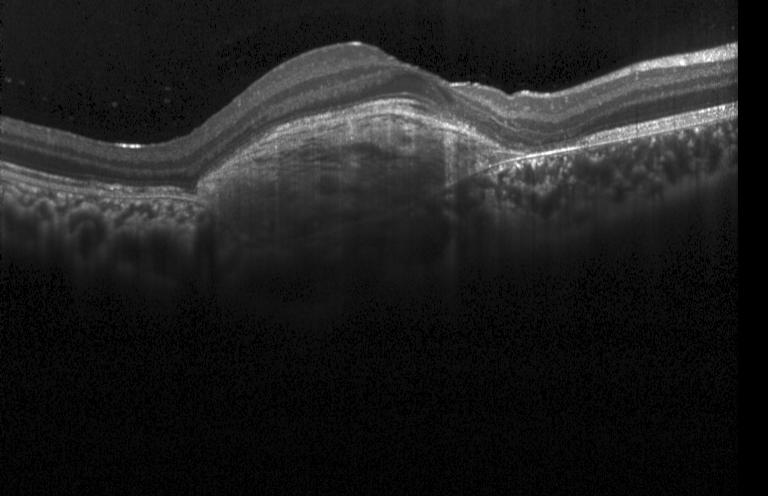 OCT B-scan — Macular OCT: a choroidal neovascular membrane.